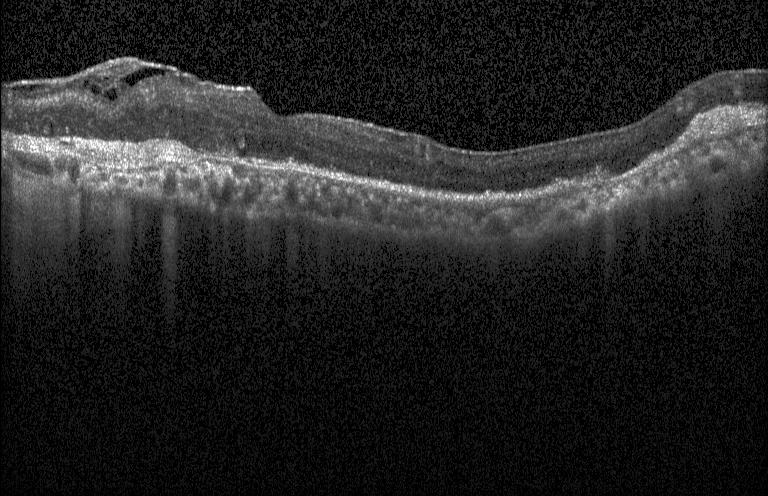

OCT line scan — Diagnosis: a choroidal neovascular membrane.